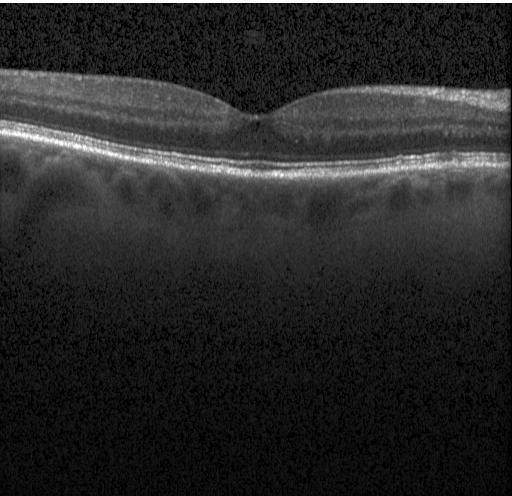
OCT B-scan · spectral-domain optical coherence tomography. Impression: no choroidal neovascularization, diabetic macular edema, or drusen.